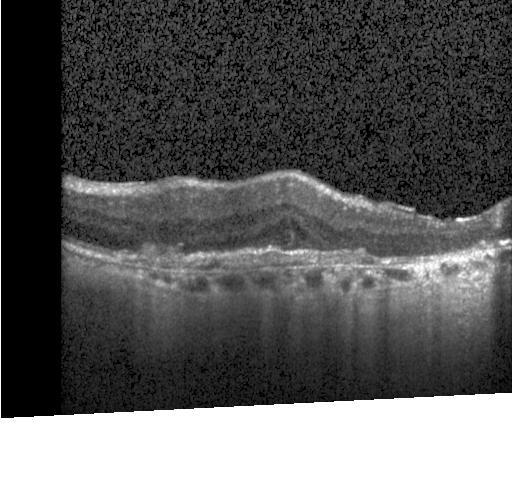
Spectral-domain optical coherence tomography. Instrument: Heidelberg Spectralis. Through the macula. OCT line scan. Impression: CNV.